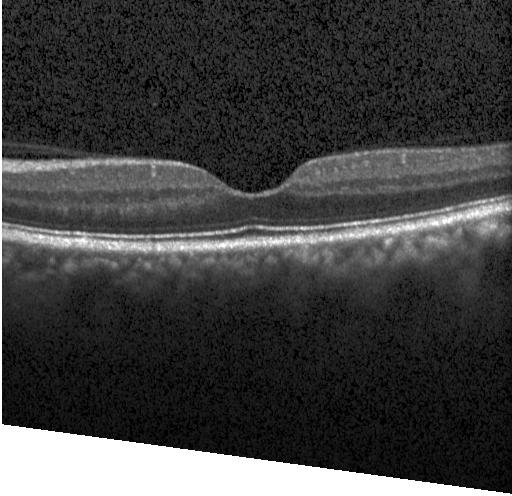
Finding: no CNV, no DME, and no drusen.